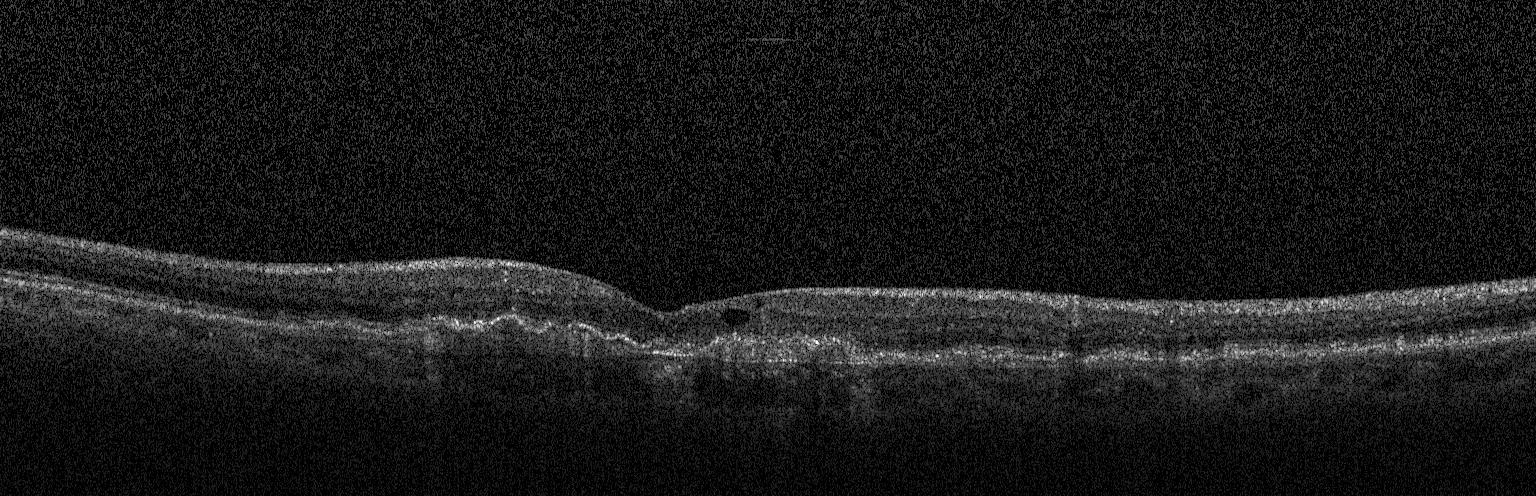
Dx: a choroidal neovascular membrane.